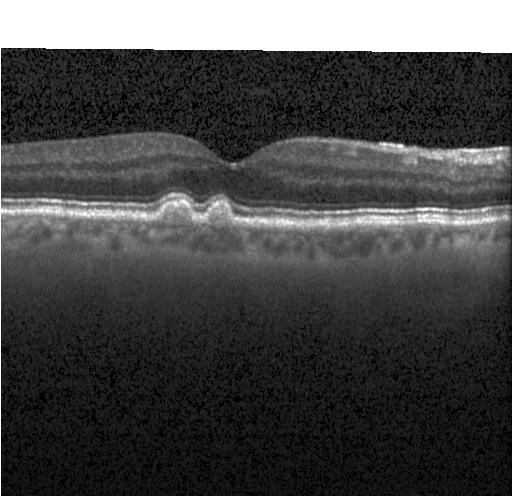

Retinal OCT B-scan. Spectral-domain optical coherence tomography. Heidelberg Spectralis OCT system.
Finding: multiple drusen.